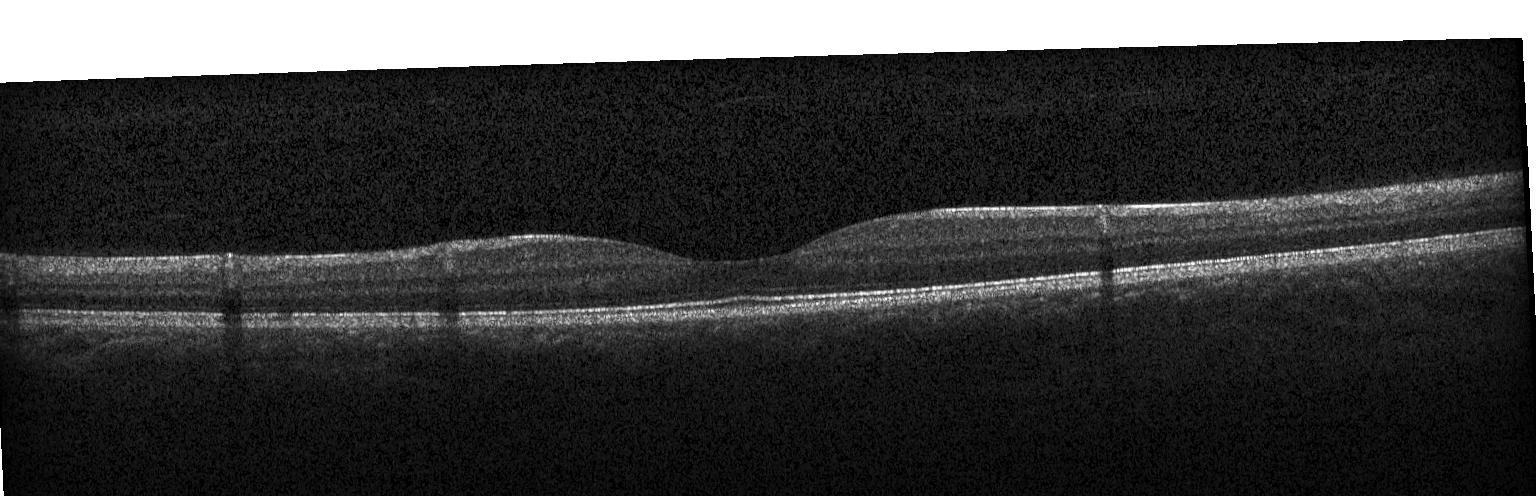

Retinal OCT cross-section · instrument: Heidelberg Spectralis · spectral-domain OCT.
Finding: neither choroidal neovascularization, diabetic macular edema, nor drusen.